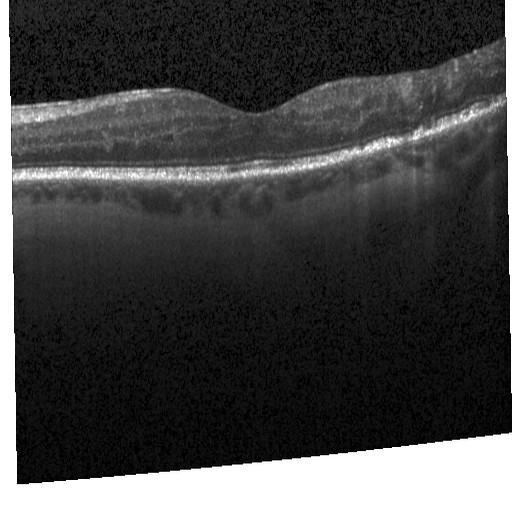 Diagnosis: diabetic macular edema.